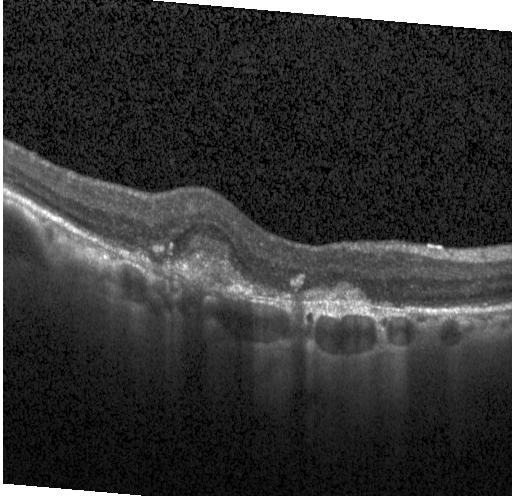
Spectral-domain OCT B-scan: choroidal neovascularization.